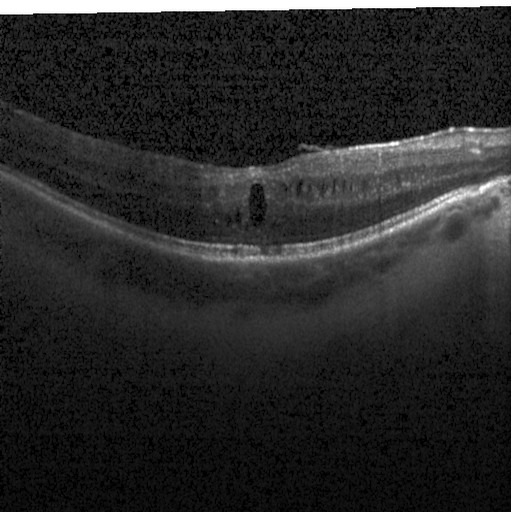

Retinal OCT cross-section; spectral-domain optical coherence tomography.
Impression: DME.